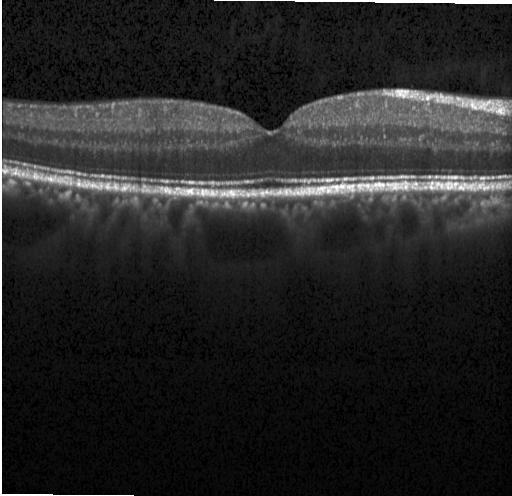

The scan shows neither CNV, DME, nor drusen.